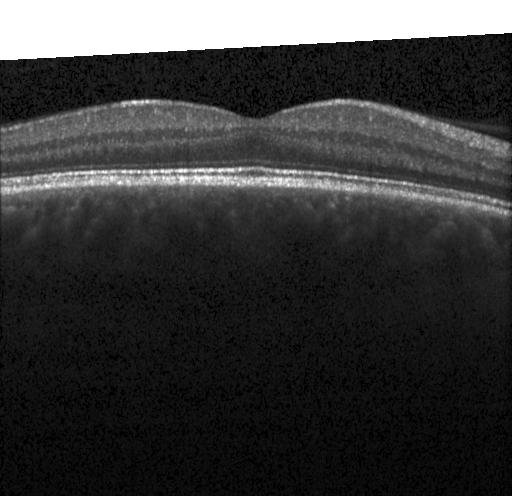

Macular OCT: no choroidal neovascularization, no diabetic macular edema, and no drusen.